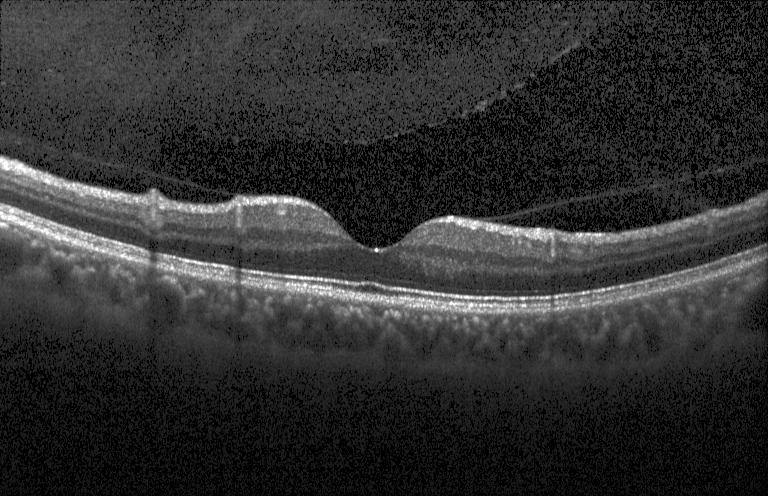
Finding: no choroidal neovascularization, no diabetic macular edema, and no drusen.